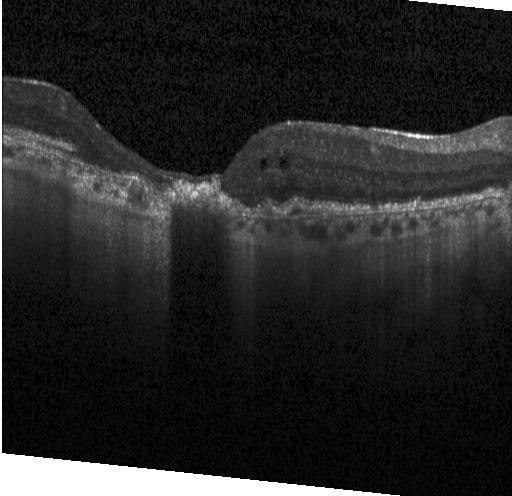

Dx: a choroidal neovascular membrane.